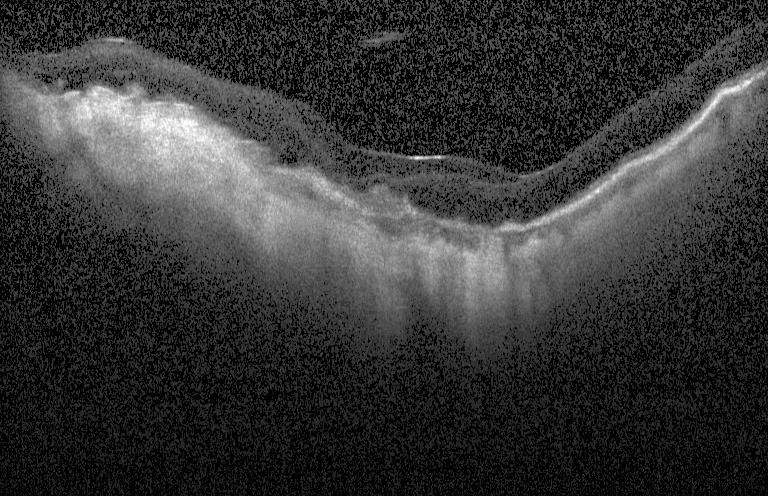

OCT B-scan. Finding: choroidal neovascularization (CNV).